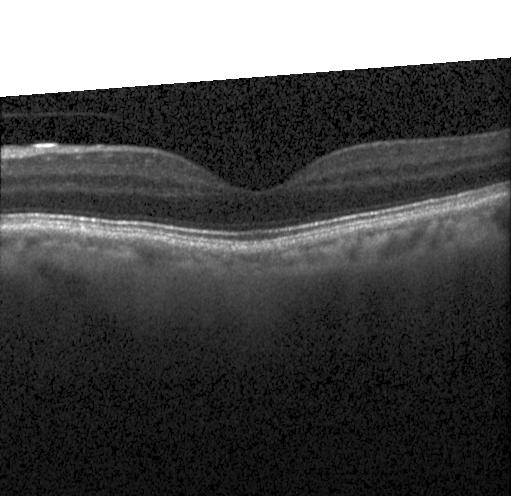
Optical coherence tomography B-scan; spectral-domain OCT; Heidelberg Spectralis OCT system; horizontal scan through the fovea.
Diagnosis: neither choroidal neovascularization, diabetic macular edema, nor drusen.